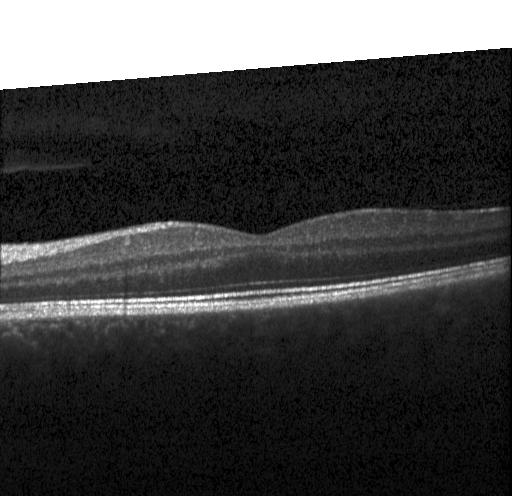
OCT line scan. The scan shows no choroidal neovascularization, no diabetic macular edema, and no drusen.